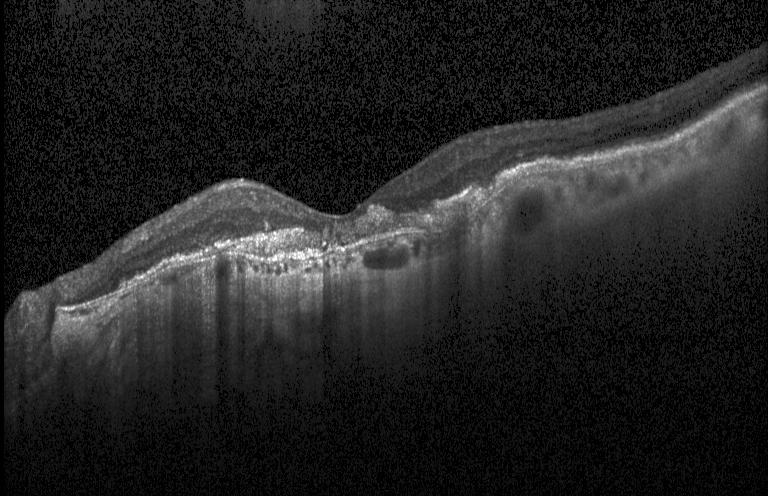

Finding: a choroidal neovascular membrane.